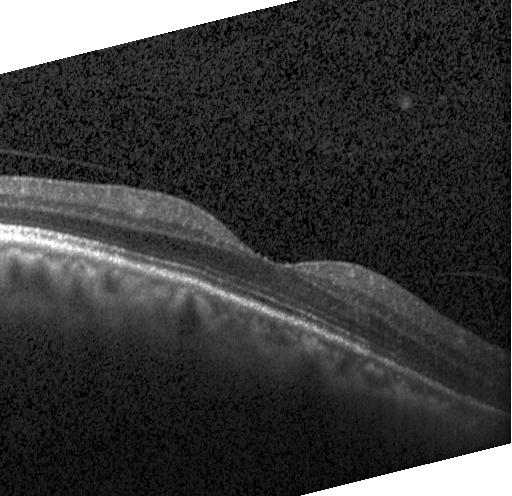

Optical coherence tomography scan, macular scan, acquired on a Heidelberg Spectralis, spectral-domain OCT.
Impression: neither choroidal neovascularization, diabetic macular edema, nor drusen.